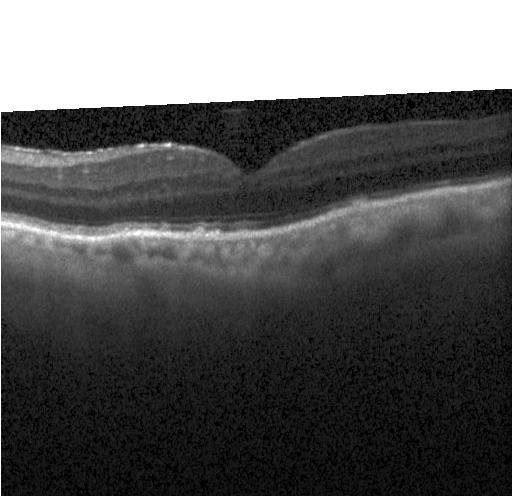
OCT finding: sub-RPE drusenoid deposits.